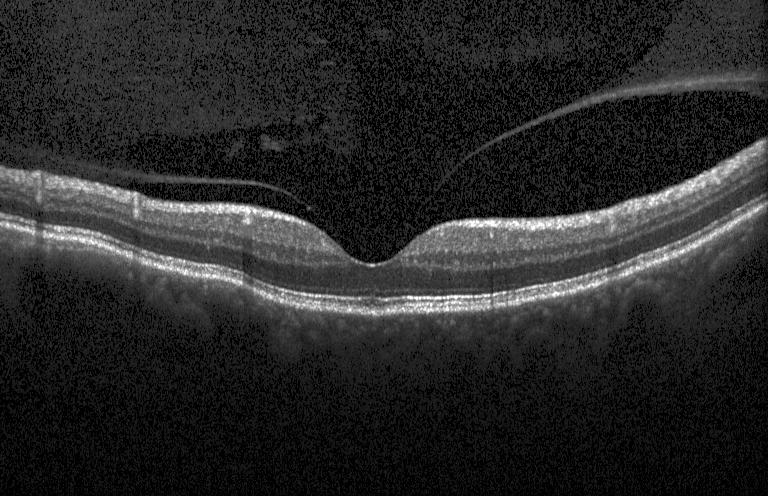

Spectral-domain optical coherence tomography · fovea-centered · OCT line scan. Macular OCT: neither choroidal neovascularization, diabetic macular edema, nor drusen.